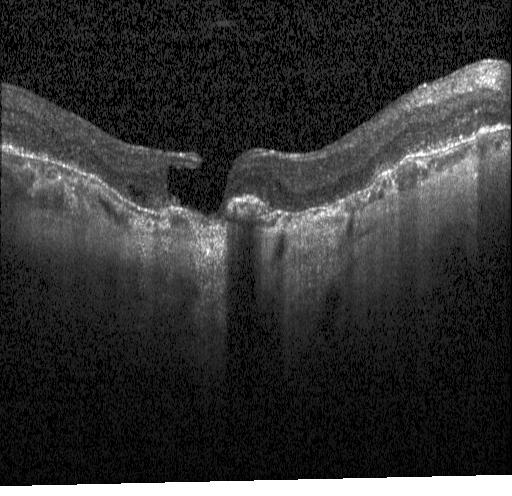

Fovea-centered. Optical coherence tomography B-scan. Heidelberg Spectralis. Impression: a choroidal neovascular membrane.